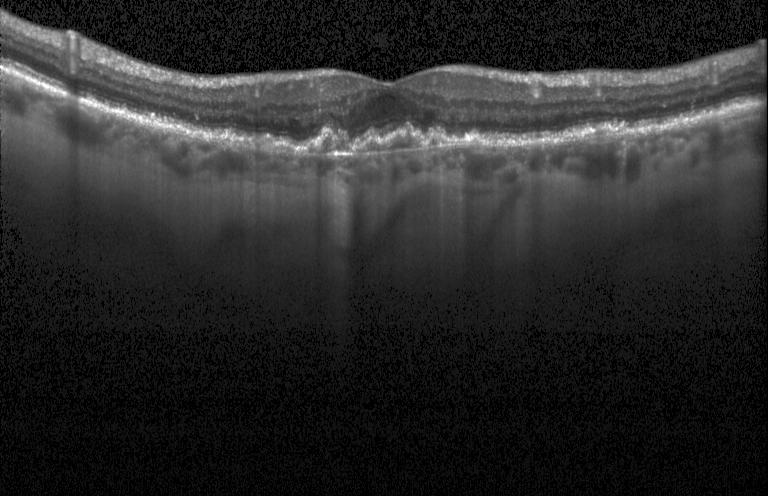
Acquired on a Heidelberg Spectralis, SD-OCT, optical coherence tomography scan. This B-scan demonstrates CNV.